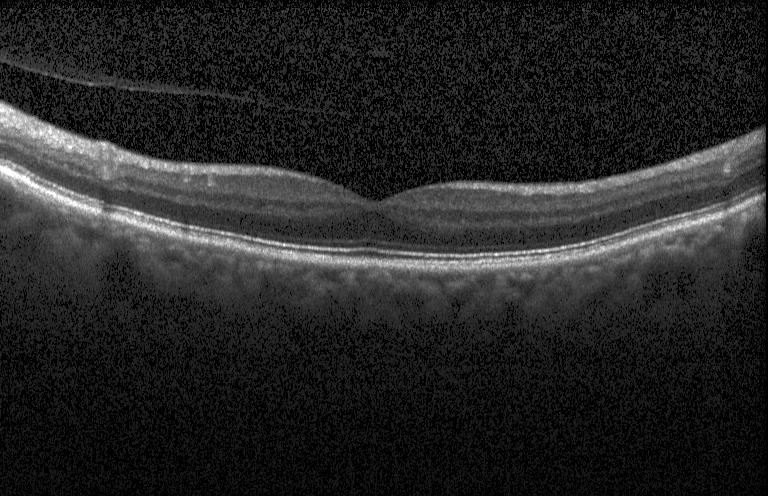 This B-scan demonstrates no CNV, DME, or drusen.